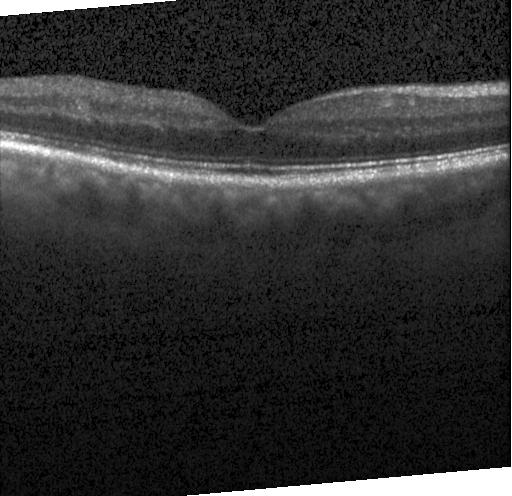 Macular OCT: no choroidal neovascularization, diabetic macular edema, or drusen.